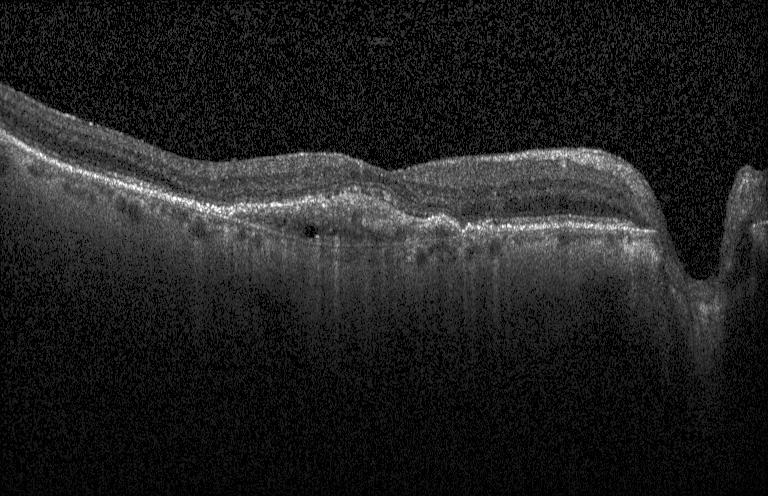
Retinal OCT cross-section.
Finding: CNV.